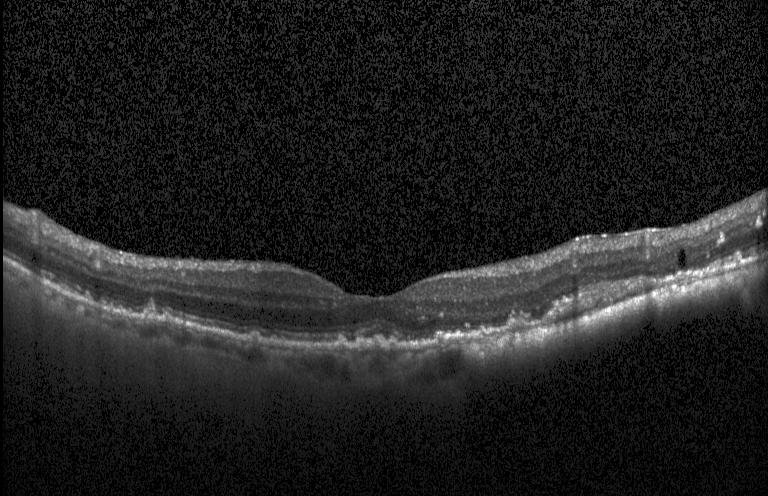

Assessment: choroidal neovascularization (CNV).